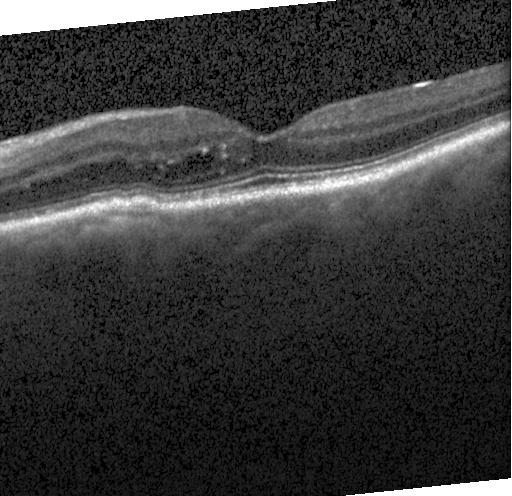
Macular OCT: diabetic macular edema (DME).